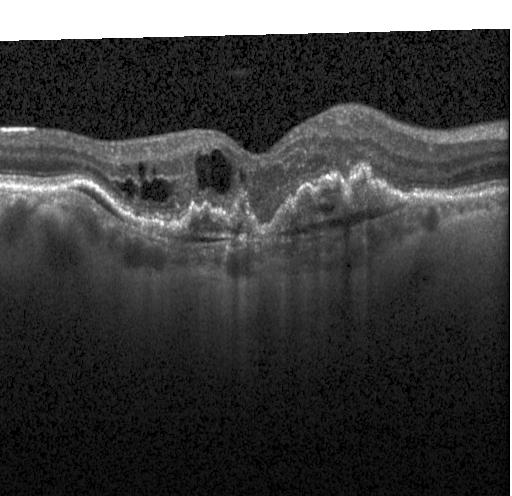

Retinal OCT cross-section — Impression: a choroidal neovascular membrane.